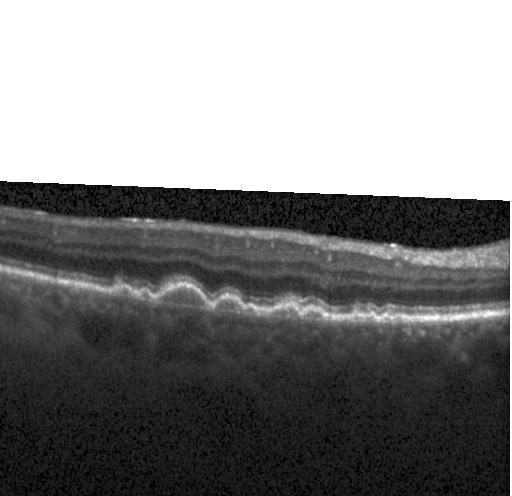
Macular scan, OCT line scan, SD-OCT. Diagnosis: a choroidal neovascular membrane.